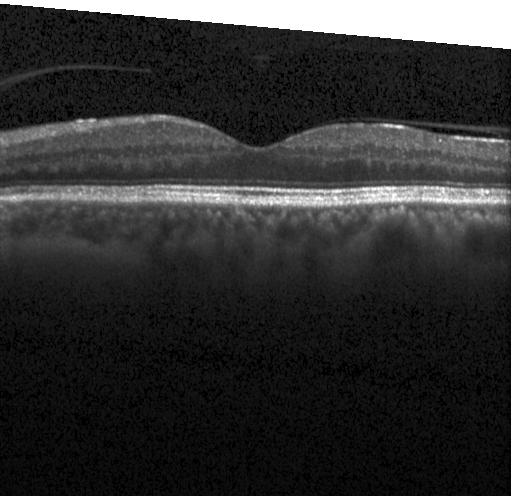 Heidelberg Spectralis. Optical coherence tomography scan. SD-OCT. Macular scan — Diagnosis: no evidence of choroidal neovascularization, diabetic macular edema, or drusen.